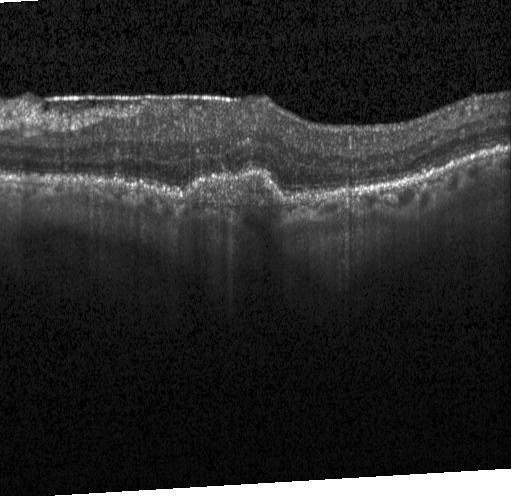
Heidelberg Spectralis. Macular scan. OCT B-scan — The scan shows choroidal neovascularization (CNV).